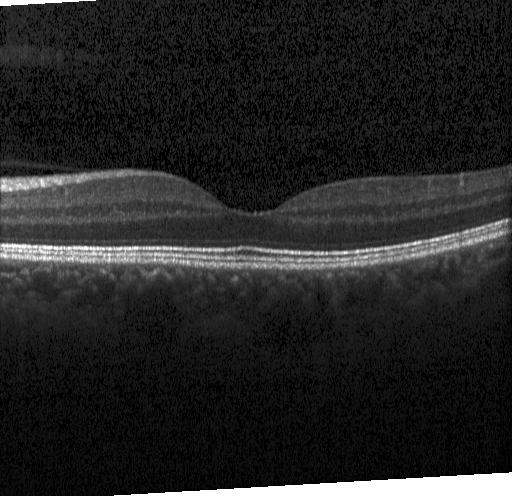
Optical coherence tomography B-scan.
Assessment: no choroidal neovascularization, no diabetic macular edema, and no drusen.